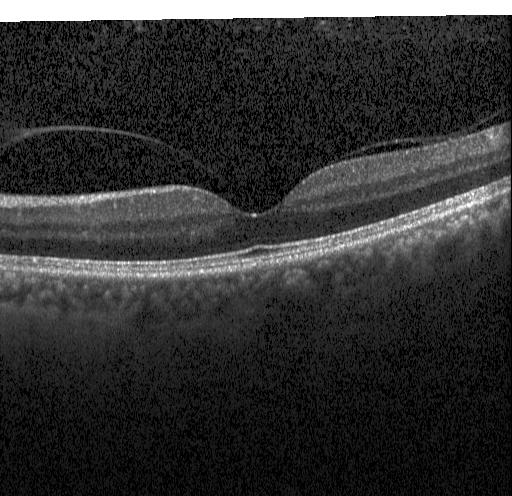 This B-scan demonstrates no CNV, DME, or drusen.